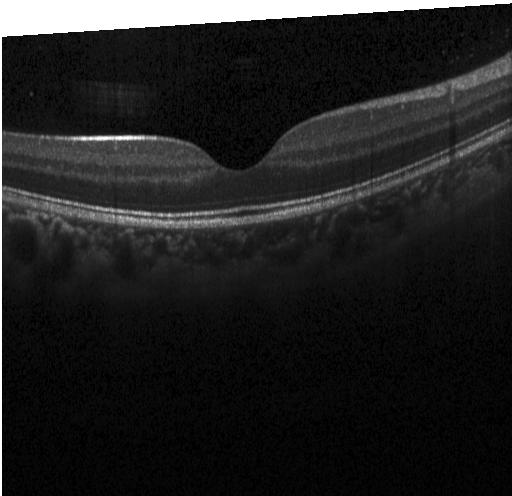

Spectral-domain OCT B-scan: no choroidal neovascularization, diabetic macular edema, or drusen.